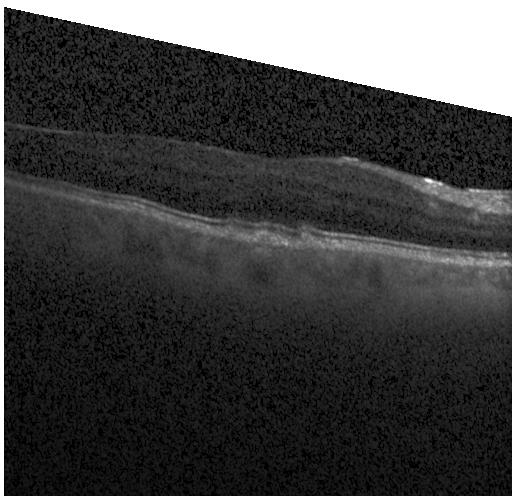
OCT line scan · Heidelberg Spectralis OCT system.
This B-scan demonstrates multiple drusen.